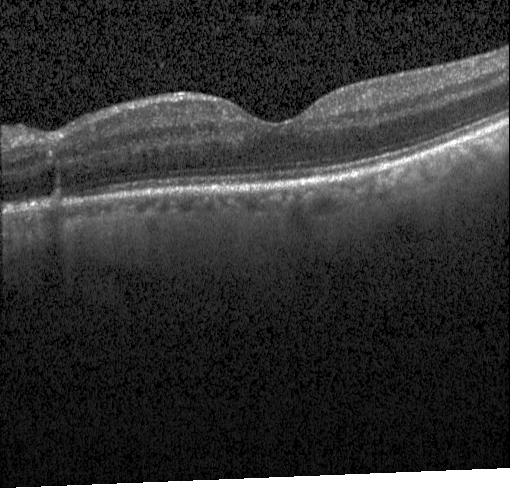
OCT B-scan. Acquired on a Heidelberg Spectralis — Impression: no evidence of choroidal neovascularization, diabetic macular edema, or drusen.